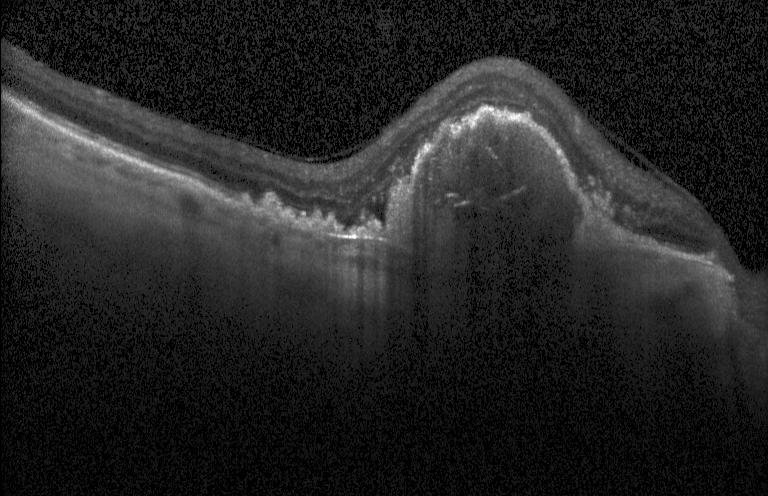

Optical coherence tomography scan, spectral-domain optical coherence tomography, Heidelberg Spectralis OCT system, macular scan — Finding: choroidal neovascularization (CNV).